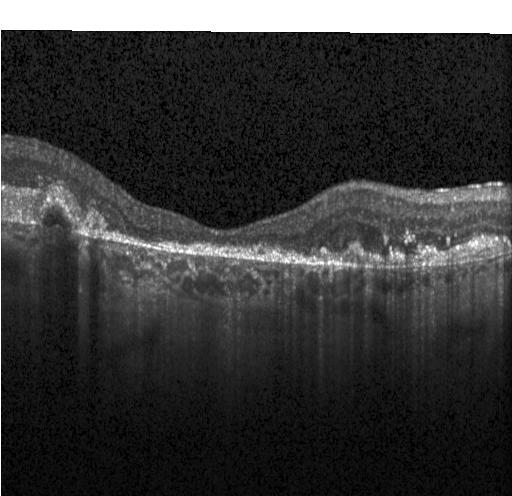

Acquired on a Heidelberg Spectralis. Horizontal scan through the fovea. Optical coherence tomography B-scan — Diagnosis: a choroidal neovascular membrane.